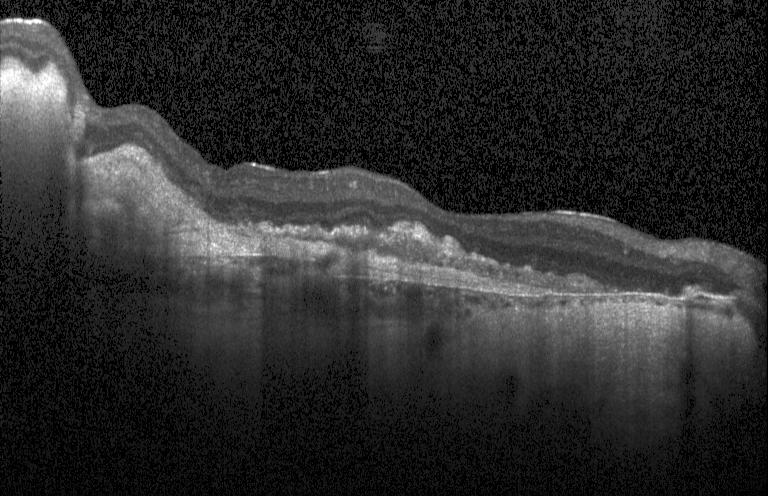

Acquired on a Heidelberg Spectralis; fovea-centered; OCT line scan; SD-OCT.
Finding: CNV.